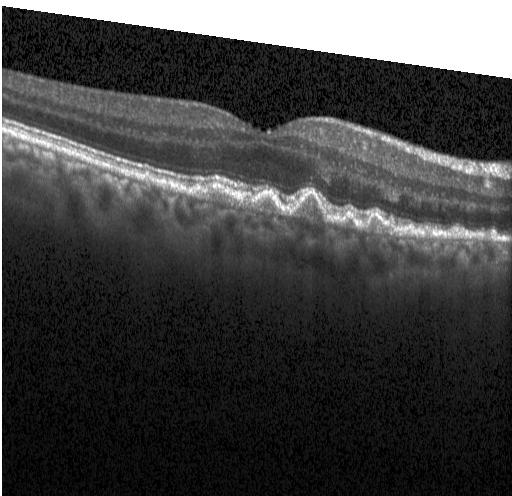

Impression: sub-RPE drusenoid deposits.